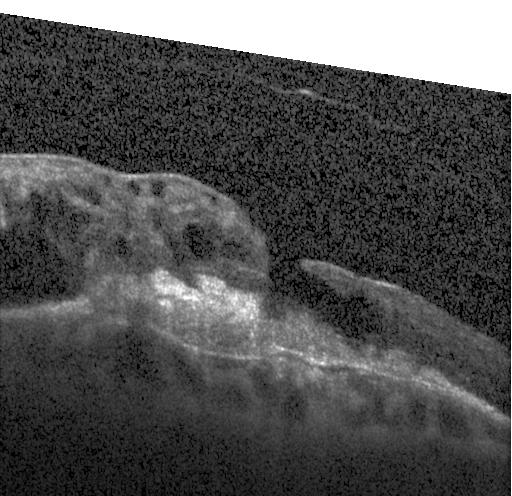

Impression: a choroidal neovascular membrane.